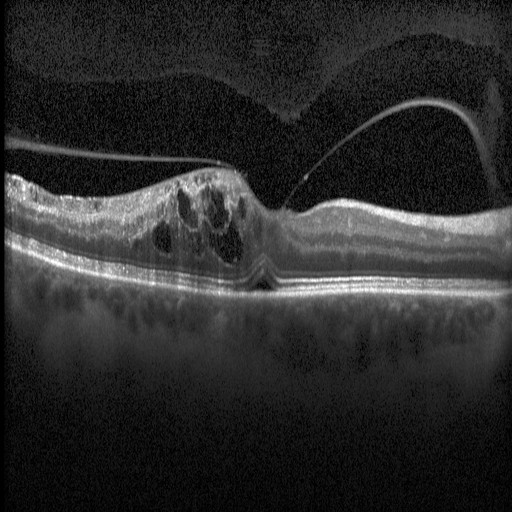
Optical coherence tomography B-scan. Finding: diabetic macular edema.